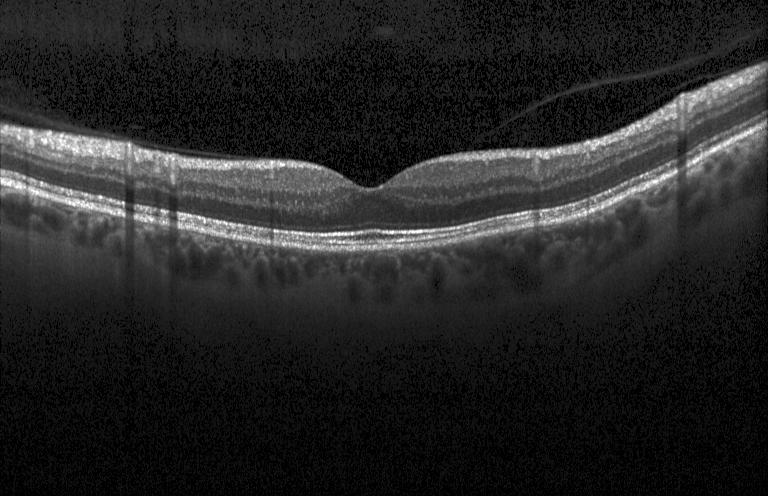 Dx: no CNV, DME, or drusen.